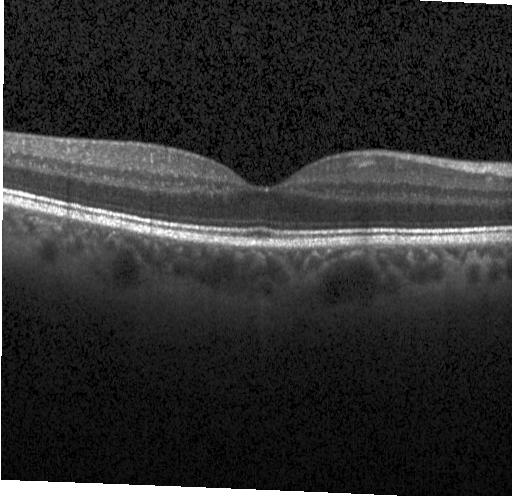
Macular OCT demonstrating no choroidal neovascularization, diabetic macular edema, or drusen.